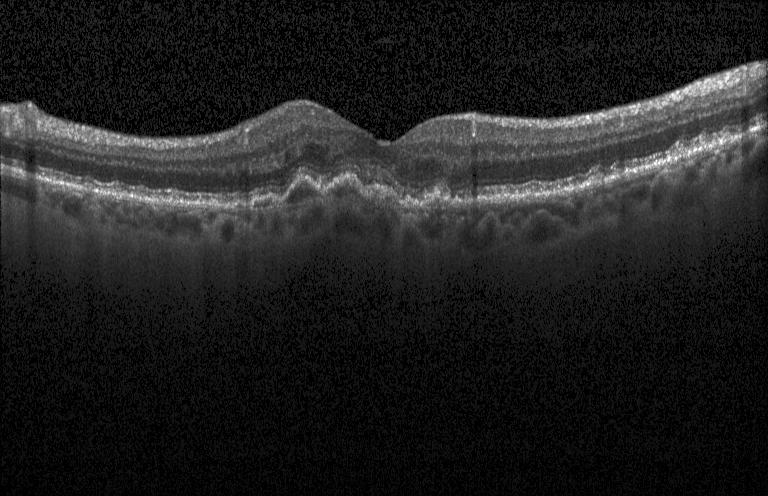
A choroidal neovascular membrane.